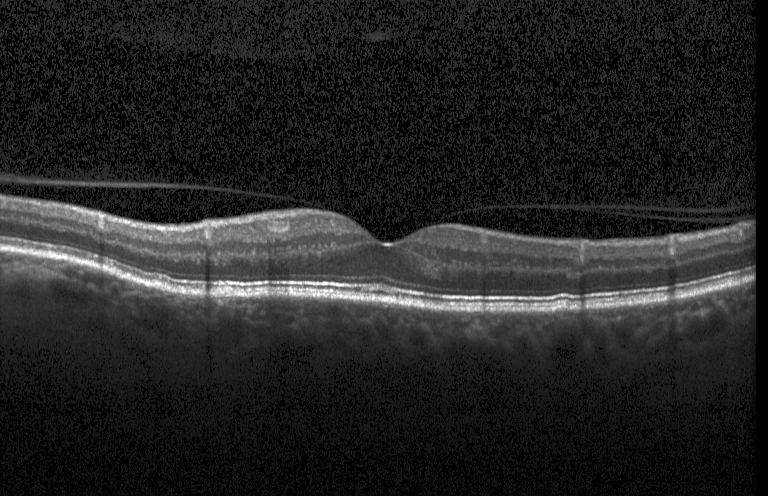

This B-scan demonstrates no CNV, no DME, and no drusen.